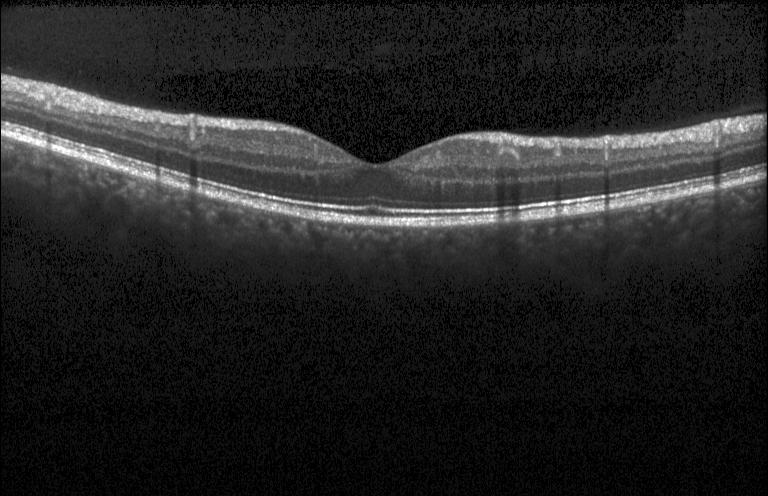
Horizontal scan through the fovea, optical coherence tomography B-scan — Assessment: neither CNV, DME, nor drusen.